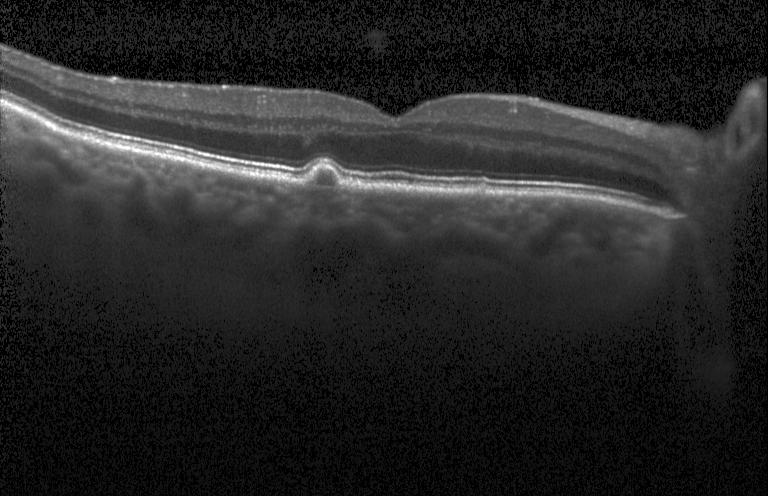

Spectral-domain optical coherence tomography. Heidelberg Spectralis. OCT B-scan. Assessment: multiple drusen.